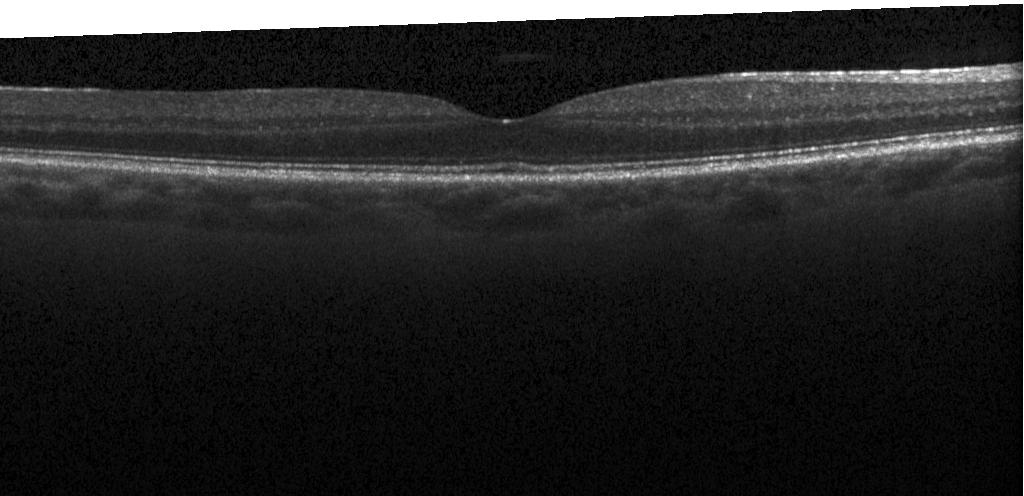 Retinal OCT cross-section.
Diagnosis: no choroidal neovascularization, no diabetic macular edema, and no drusen.